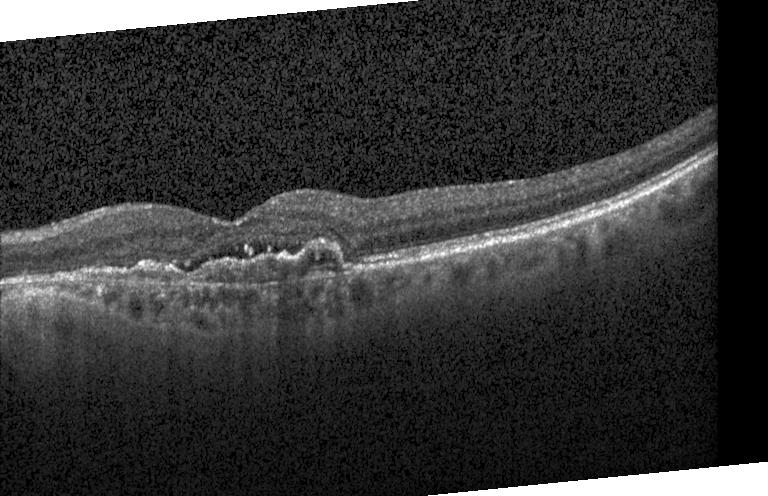

Optical coherence tomography B-scan. Diagnosis: a choroidal neovascular membrane.